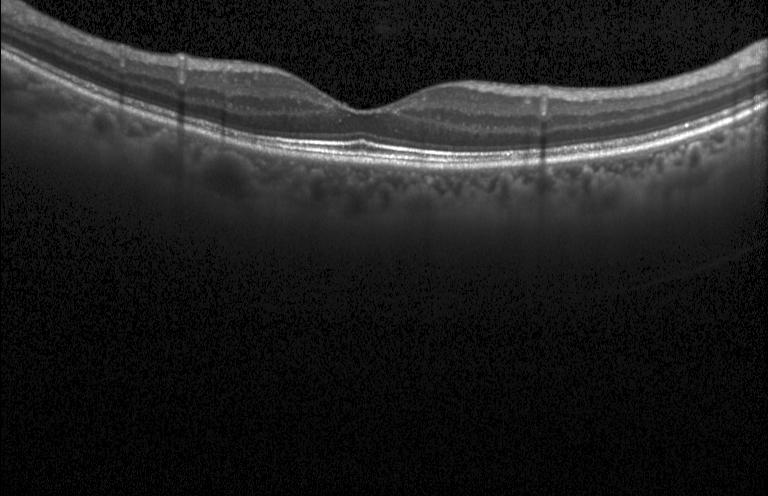

OCT B-scan showing no evidence of choroidal neovascularization, diabetic macular edema, or drusen.